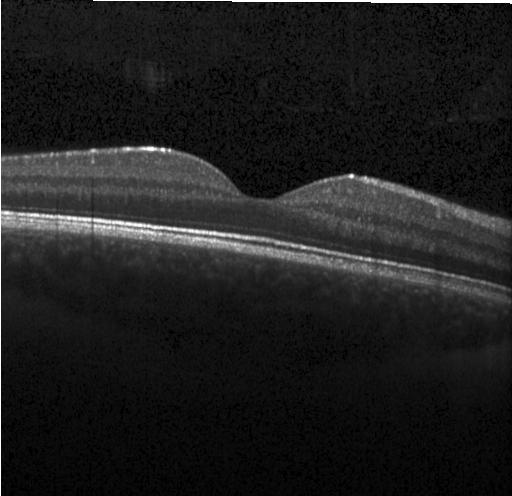 Retinal OCT B-scan
Finding: no choroidal neovascularization, no diabetic macular edema, and no drusen.